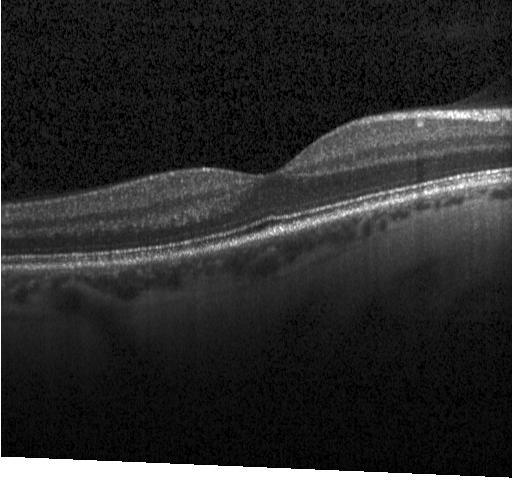 Retinal OCT B-scan, acquired on a Heidelberg Spectralis, SD-OCT
Diagnosis: no evidence of choroidal neovascularization, diabetic macular edema, or drusen.